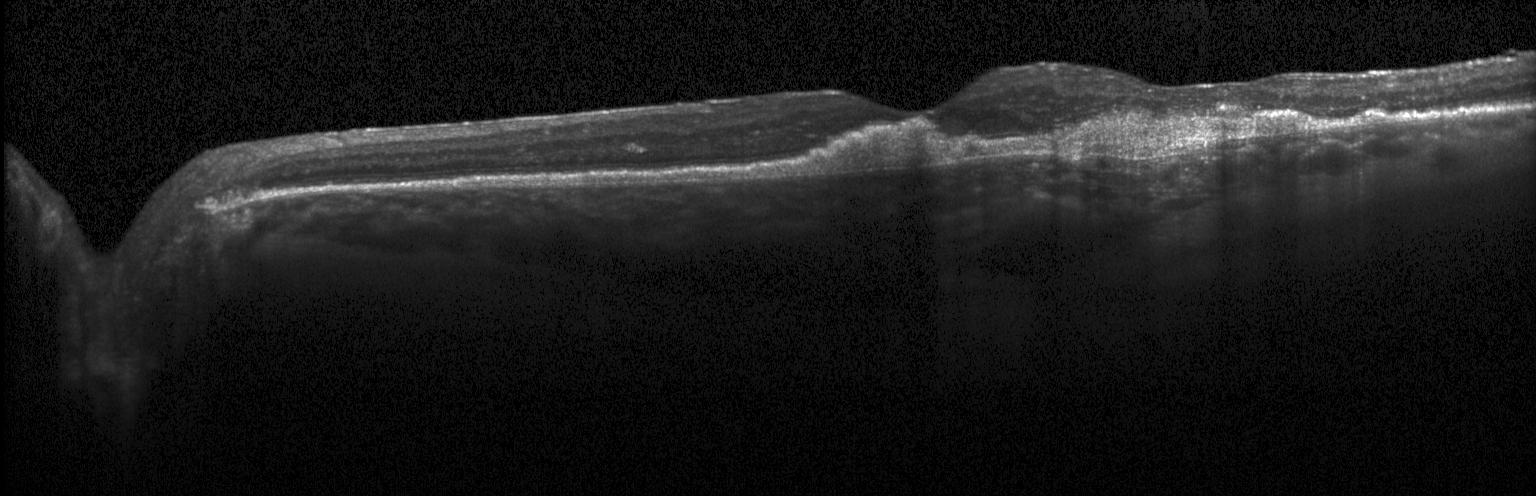 OCT scan showing choroidal neovascularization.